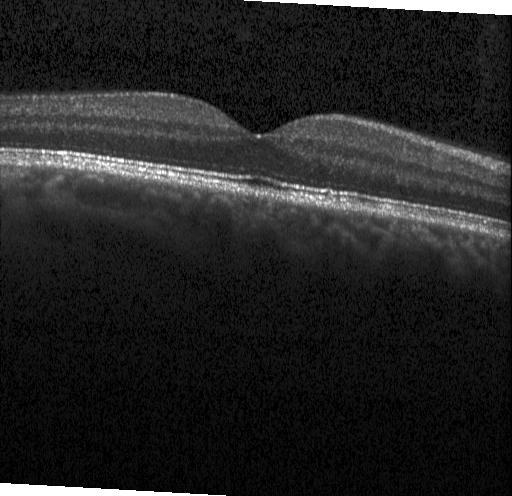
This B-scan demonstrates neither choroidal neovascularization, diabetic macular edema, nor drusen.